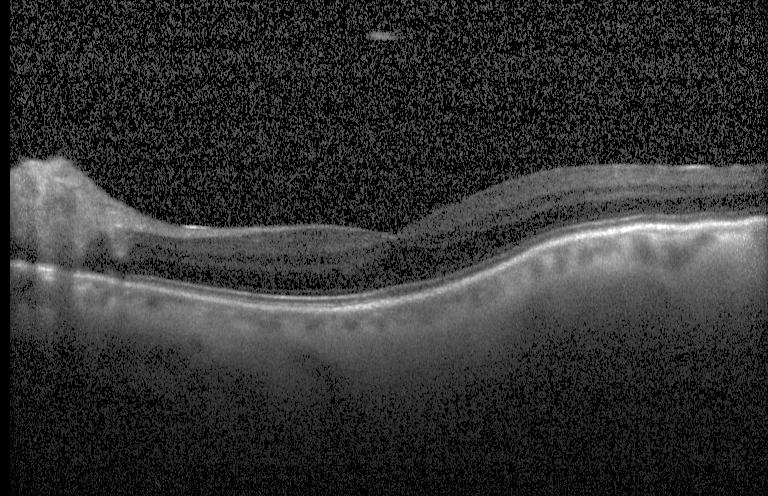

Spectral-domain optical coherence tomography. Retinal OCT cross-section. Through the macula. Finding: no CNV, DME, or drusen.